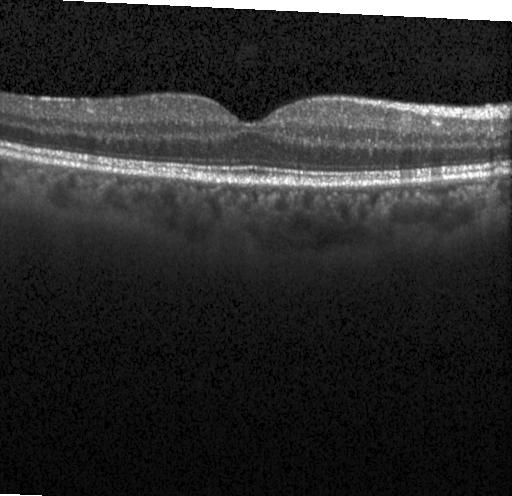 Spectral-domain optical coherence tomography. Optical coherence tomography scan. Instrument: Heidelberg Spectralis — Dx: no choroidal neovascularization, diabetic macular edema, or drusen.